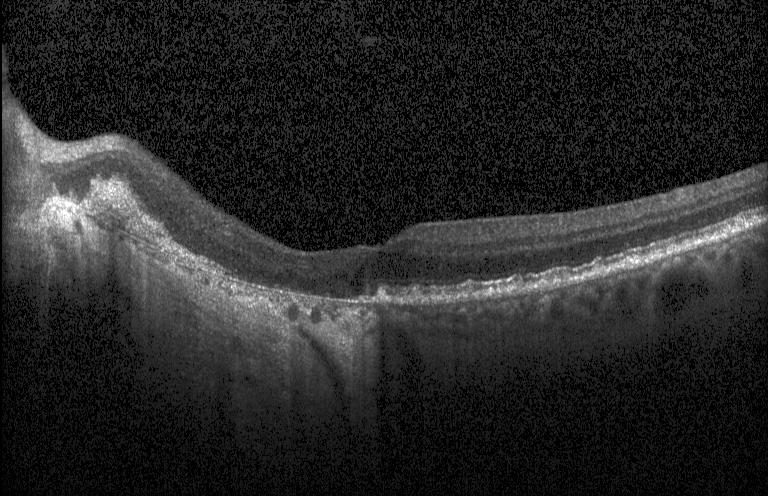

OCT line scan — OCT finding: CNV.